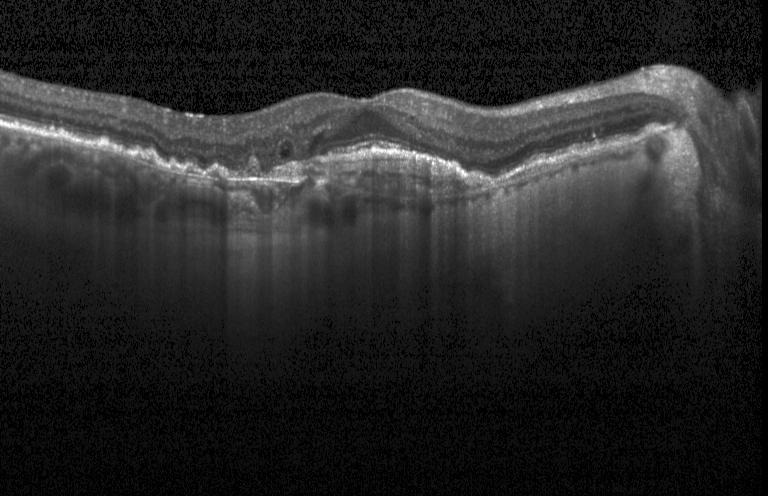

Retinal OCT cross-section, instrument: Heidelberg Spectralis, horizontal scan through the fovea, spectral-domain OCT. Dx: a choroidal neovascular membrane.